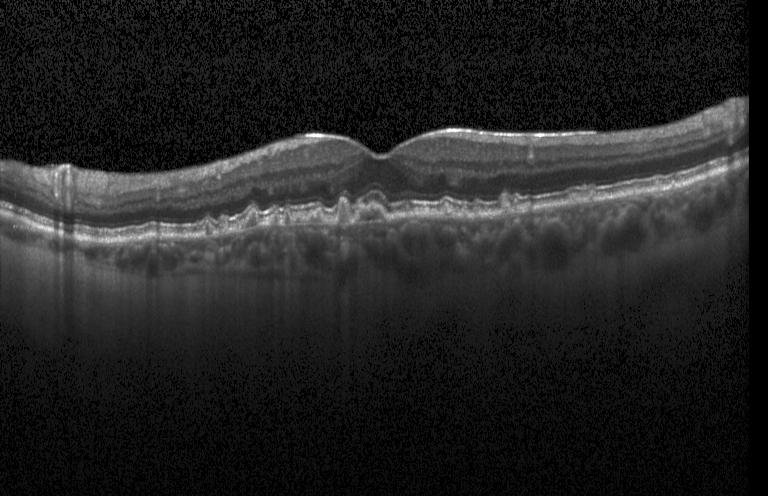

Impression: multiple drusen.